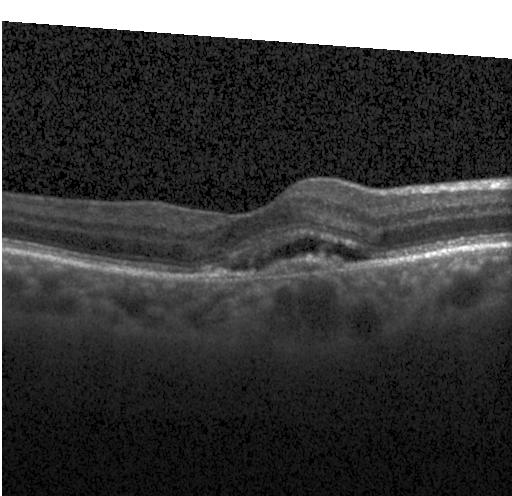
Retinal OCT B-scan · fovea-centered · instrument: Heidelberg Spectralis
Diagnosis: a choroidal neovascular membrane.